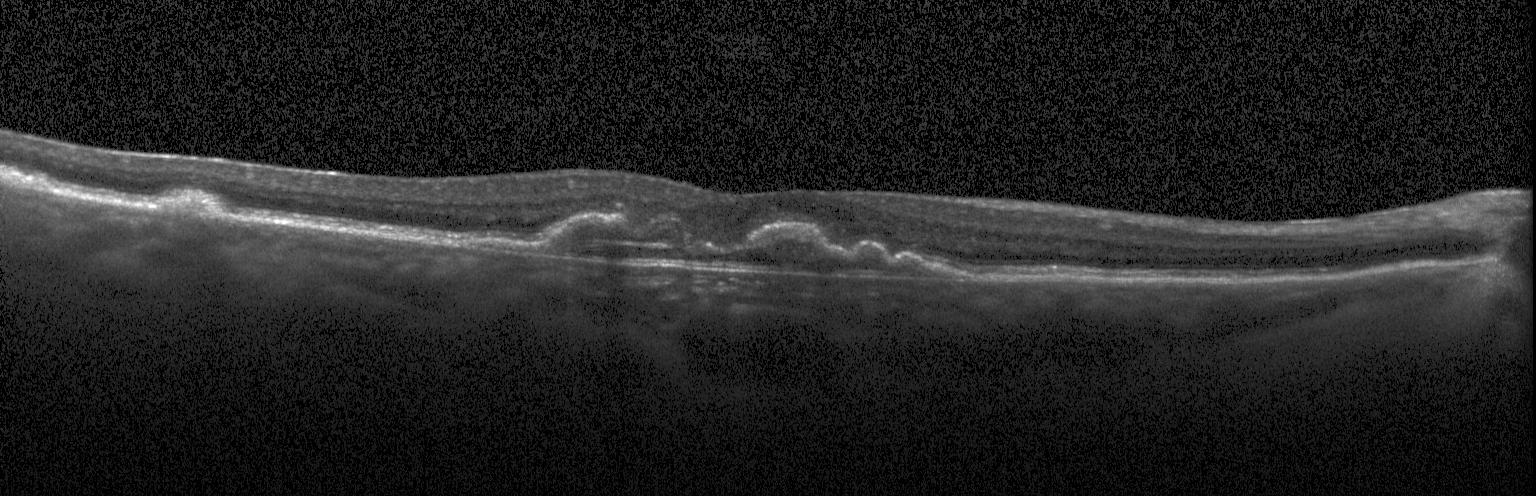 Fovea-centered · Heidelberg Spectralis · retinal OCT B-scan — Dx: a choroidal neovascular membrane.